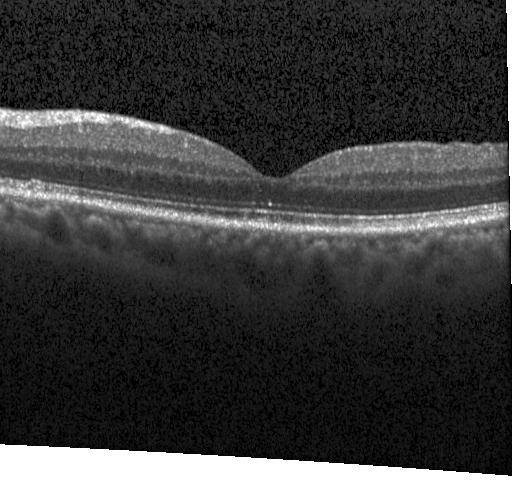

Spectral-domain optical coherence tomography; optical coherence tomography scan.
Diagnosis: no evidence of choroidal neovascularization, diabetic macular edema, or drusen.